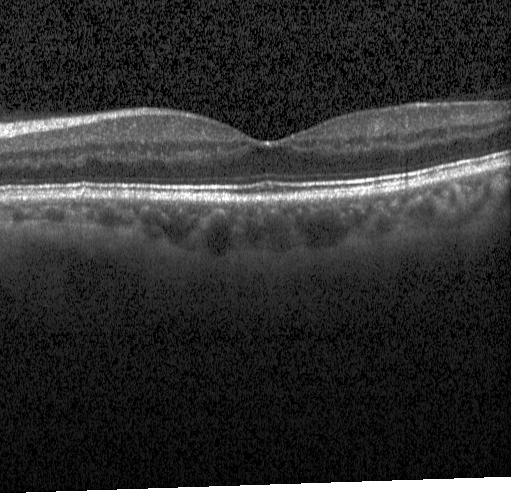 Impression: no choroidal neovascularization, diabetic macular edema, or drusen.